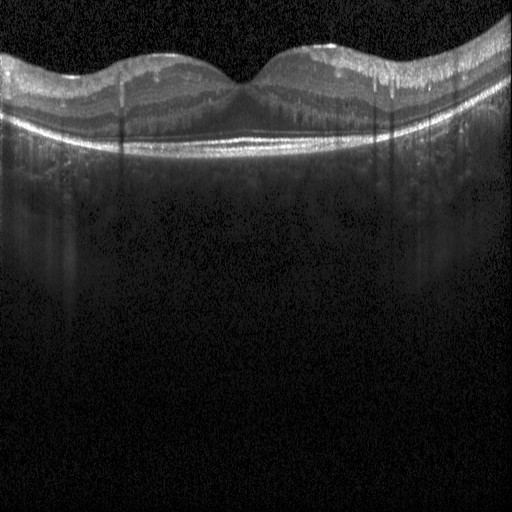
OCT line scan; Heidelberg Spectralis; centered on the fovea
This B-scan demonstrates diabetic macular edema (DME).